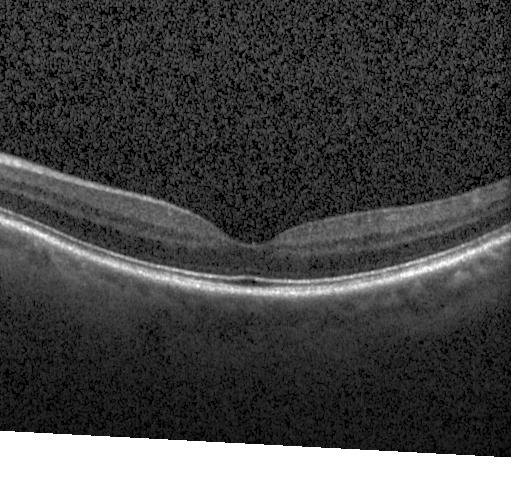
Macular OCT demonstrating no evidence of choroidal neovascularization, diabetic macular edema, or drusen.